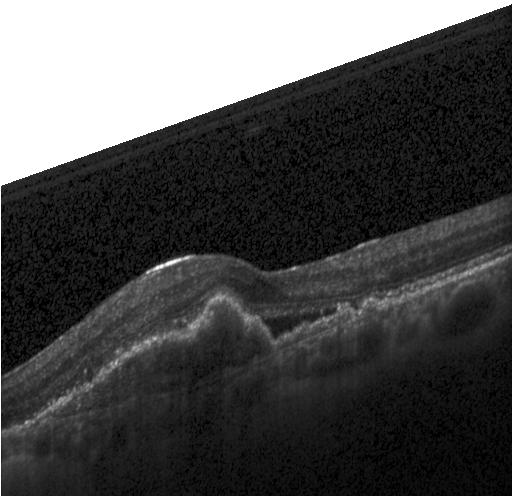
Retinal OCT B-scan
OCT finding: choroidal neovascularization (CNV).